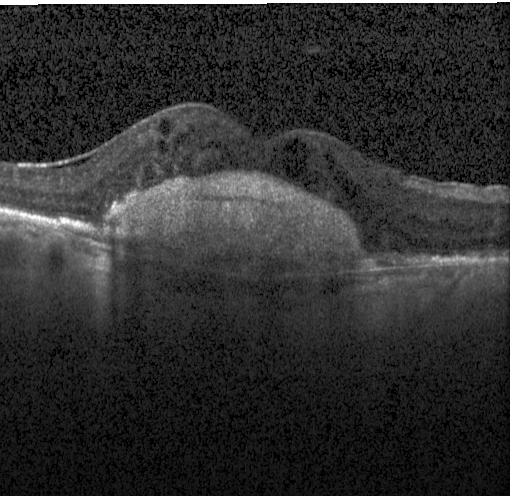 Impression: a choroidal neovascular membrane.